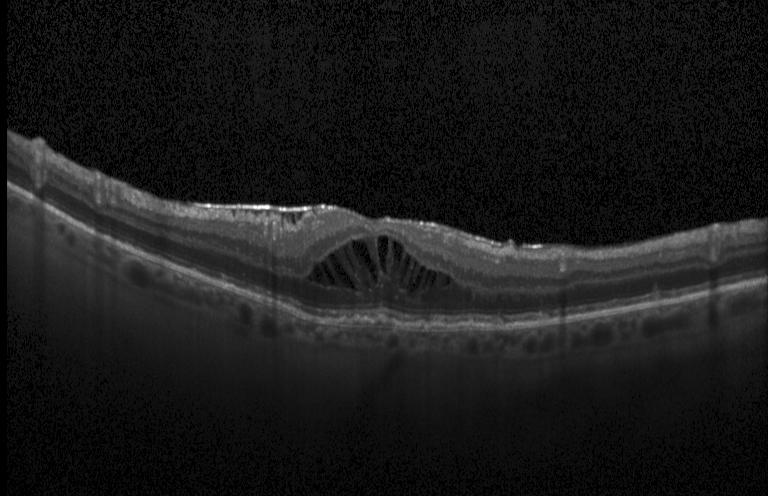

Spectral-domain OCT · acquired on a Heidelberg Spectralis · retinal OCT cross-section · through the macula. Impression: DME.